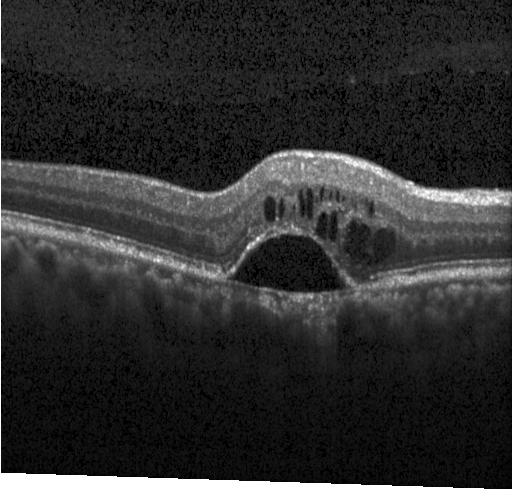 Spectral-domain OCT; OCT B-scan; Heidelberg Spectralis.
OCT finding: a choroidal neovascular membrane.